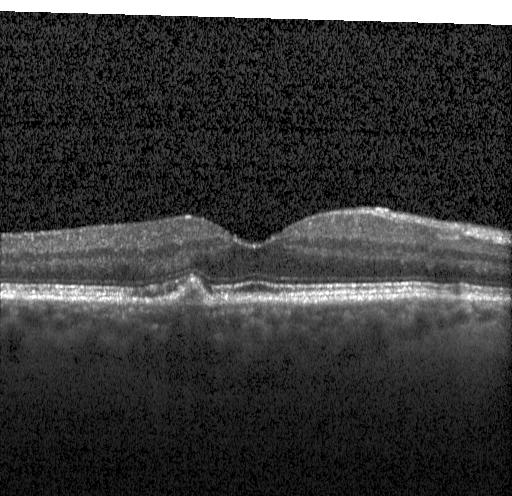
Macular scan. OCT line scan. Diagnosis: sub-RPE drusenoid deposits.